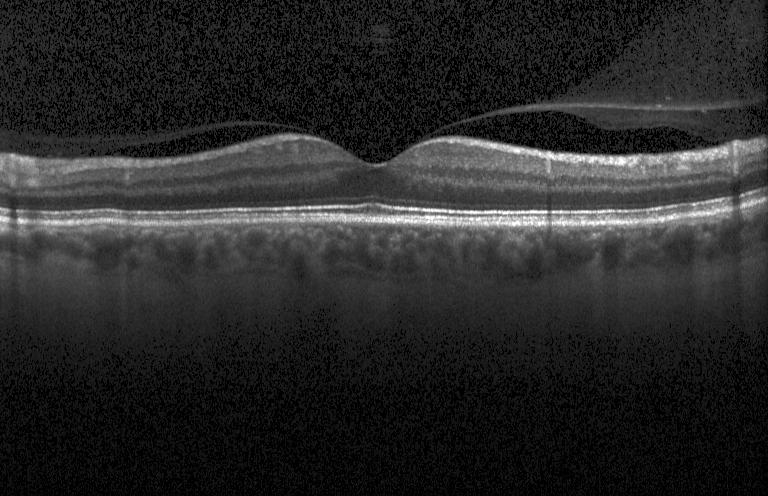
Finding: no evidence of choroidal neovascularization, diabetic macular edema, or drusen.